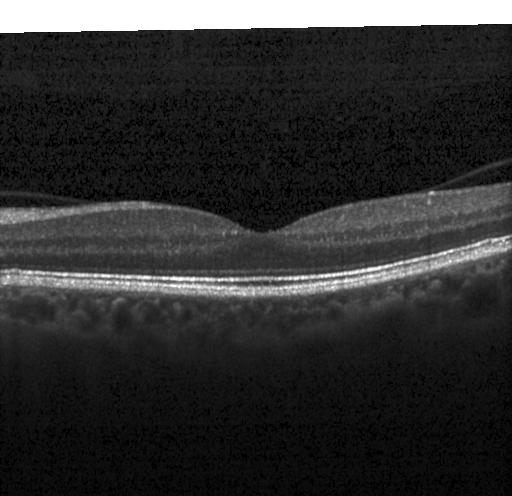

Dx: no CNV, DME, or drusen.